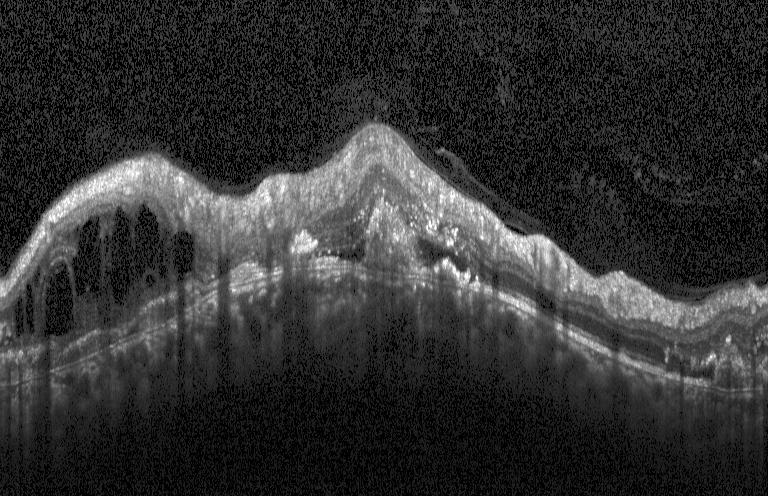 Optical coherence tomography scan. Instrument: Heidelberg Spectralis
Impression: a choroidal neovascular membrane.